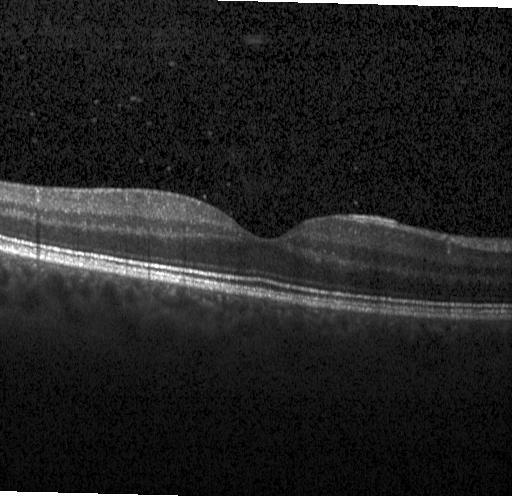

Optical coherence tomography B-scan · Heidelberg Spectralis OCT system · horizontal scan through the fovea
OCT finding: neither choroidal neovascularization, diabetic macular edema, nor drusen.